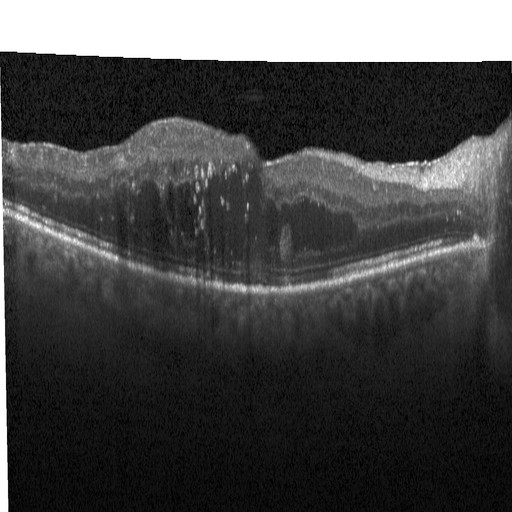 Retinal OCT cross-section. The scan shows DME.